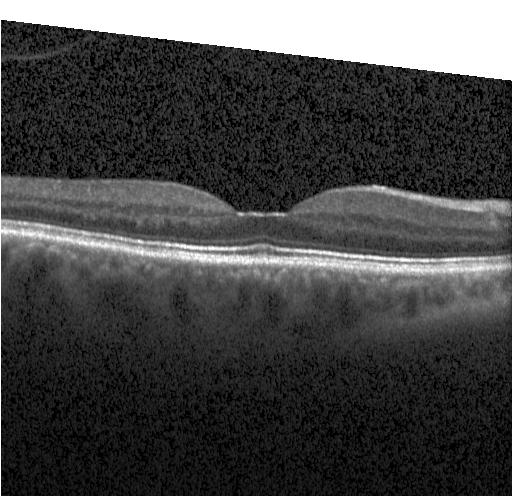 Centered on the fovea, retinal OCT cross-section, instrument: Heidelberg Spectralis, spectral-domain OCT
Dx: neither CNV, DME, nor drusen.